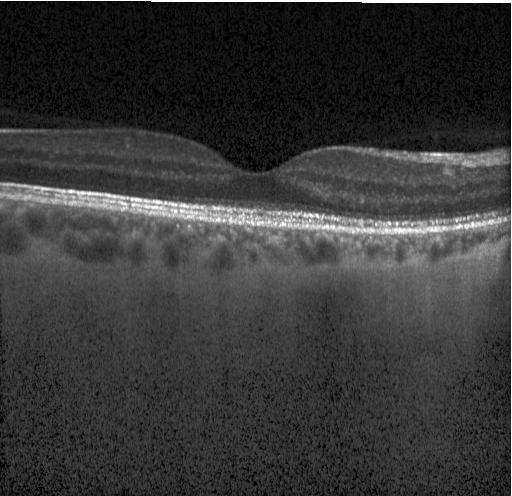

Optical coherence tomography scan; spectral-domain optical coherence tomography
The scan shows no CNV, no DME, and no drusen.